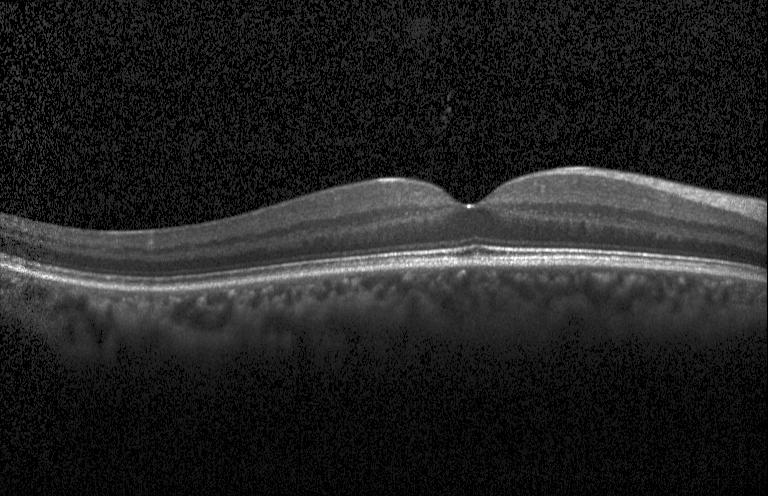

OCT finding: neither CNV, DME, nor drusen.